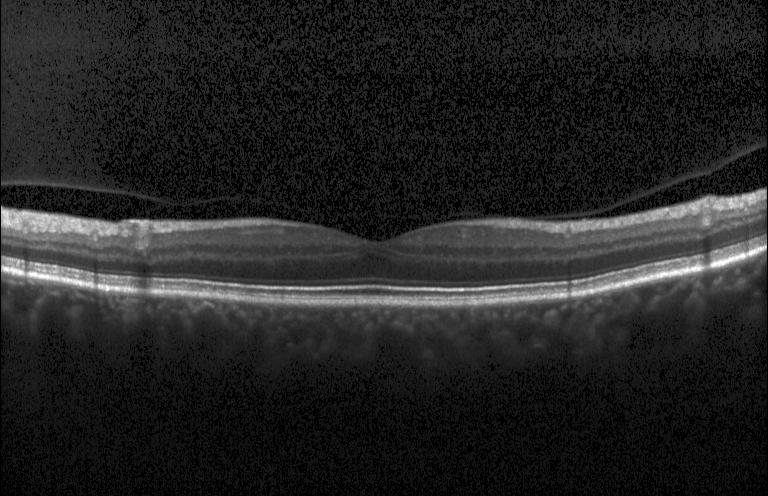 Optical coherence tomography B-scan
Dx: no evidence of CNV, DME, or drusen.